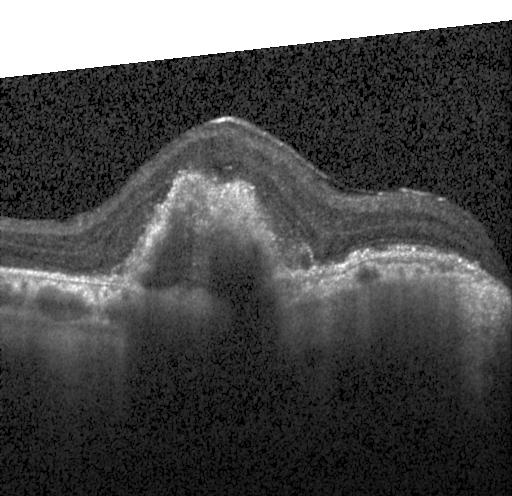 Spectral-domain OCT; OCT line scan; centered on the fovea — Assessment: a choroidal neovascular membrane.